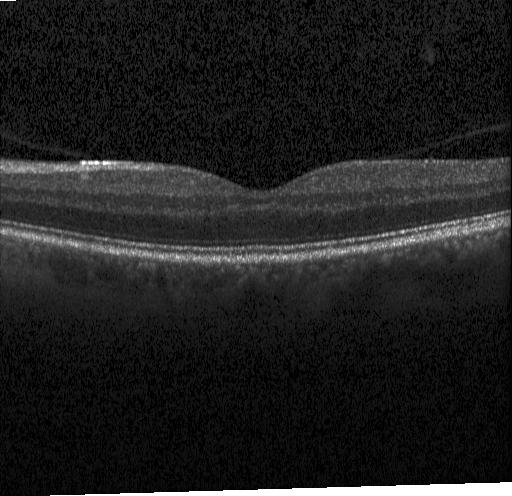
Impression: no evidence of CNV, DME, or drusen.